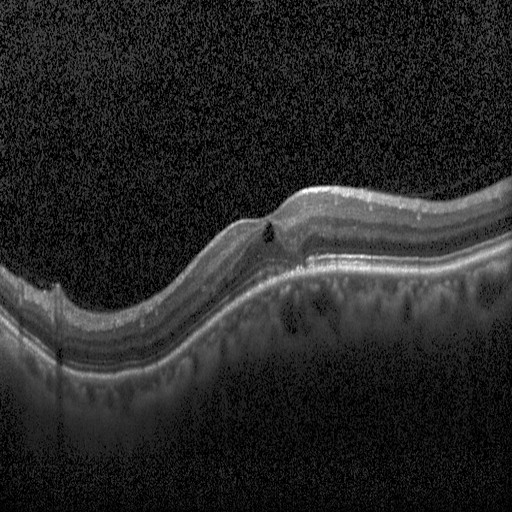 Finding: diabetic macular edema (DME).